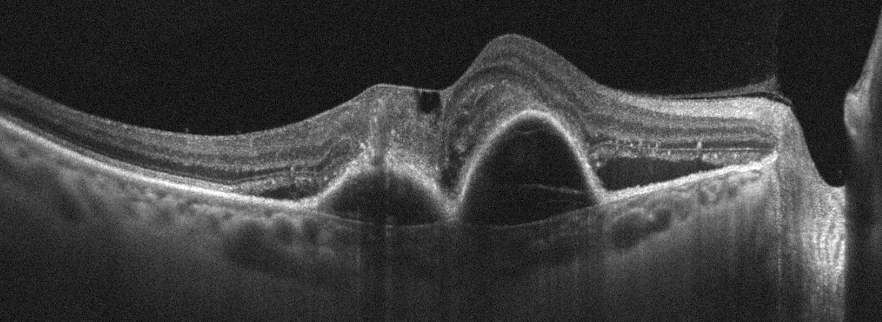

Retinal OCT cross-section
Macular OCT: age-related macular degeneration (AMD).